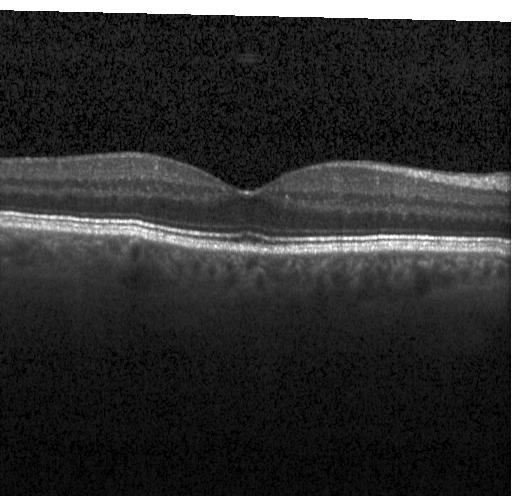
Heidelberg Spectralis OCT system, optical coherence tomography scan, through the macula
Finding: no evidence of choroidal neovascularization, diabetic macular edema, or drusen.